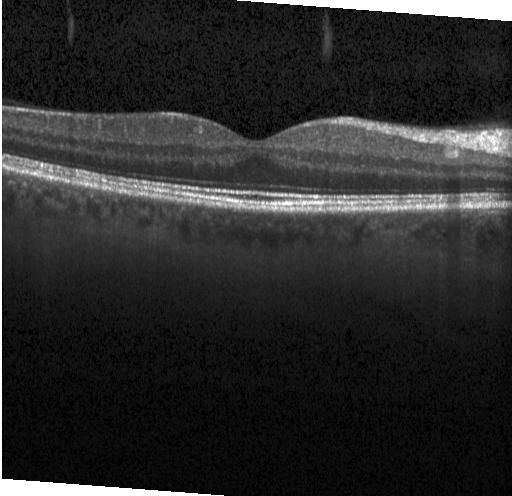 Acquired on a Heidelberg Spectralis · OCT B-scan.
The scan shows no choroidal neovascularization, diabetic macular edema, or drusen.